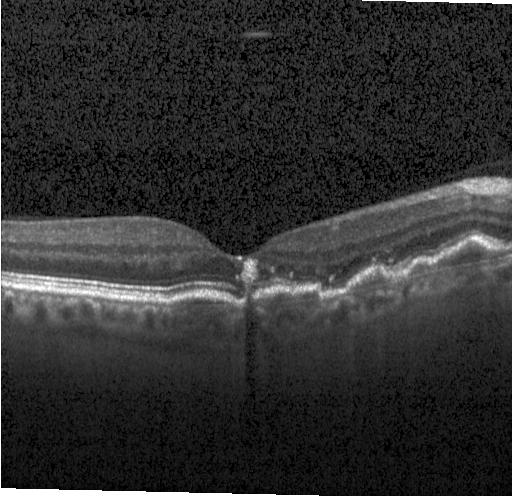
Impression: CNV.